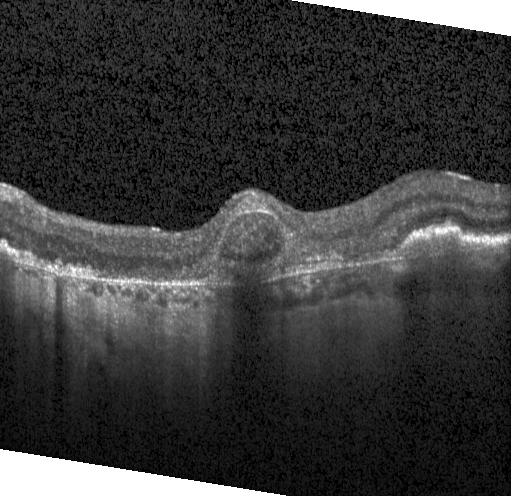
SD-OCT, optical coherence tomography B-scan, Heidelberg Spectralis OCT system.
Macular OCT: a choroidal neovascular membrane.